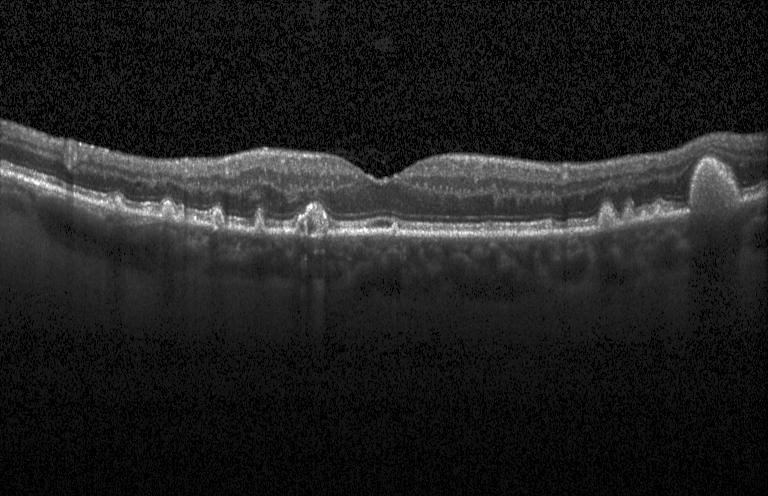
Spectral-domain OCT B-scan: multiple drusen.